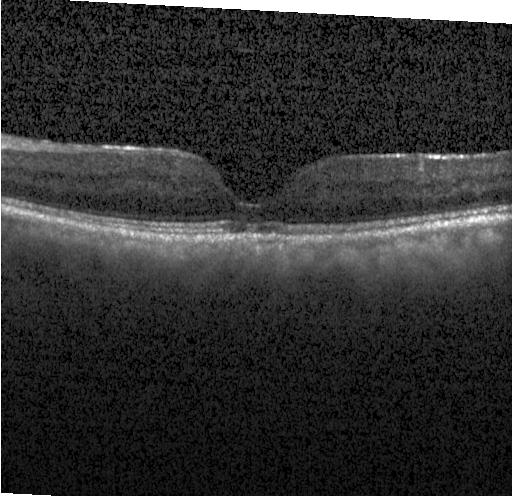

OCT finding: neither CNV, DME, nor drusen.